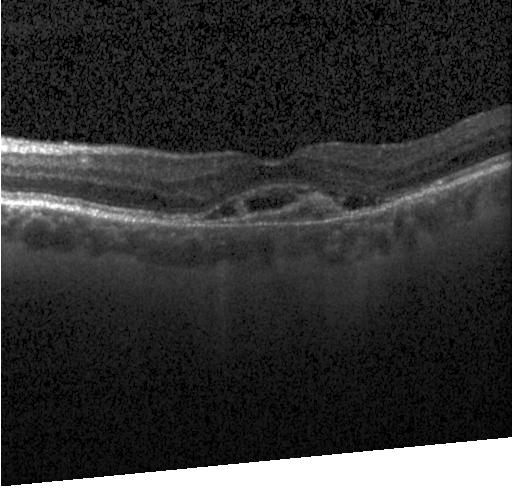
Impression: CNV.